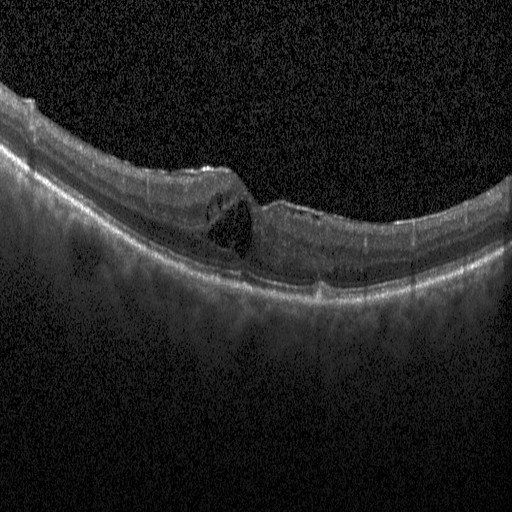
Optical coherence tomography B-scan, macular scan, SD-OCT, Heidelberg Spectralis OCT system. Finding: DME.